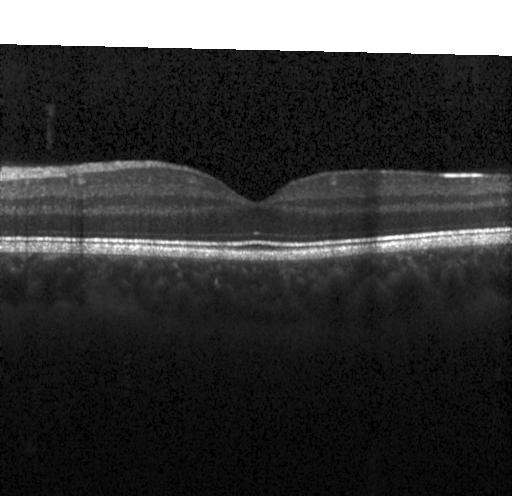
Fovea-centered · optical coherence tomography B-scan.
Finding: no evidence of choroidal neovascularization, diabetic macular edema, or drusen.